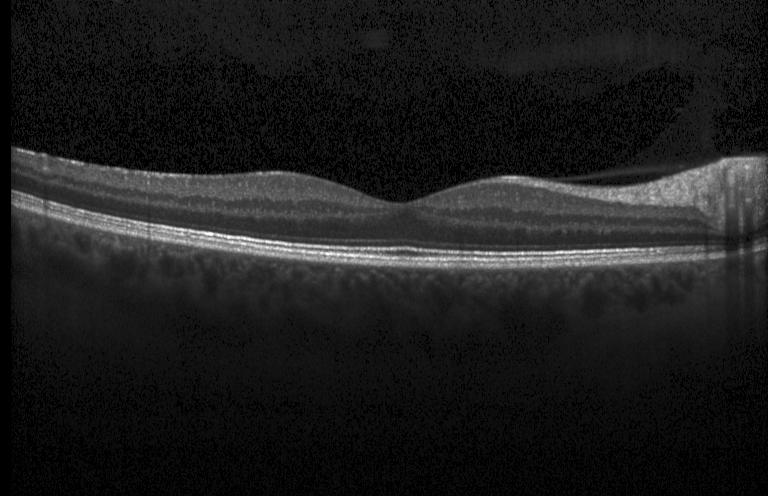 Macular OCT: no CNV, DME, or drusen.